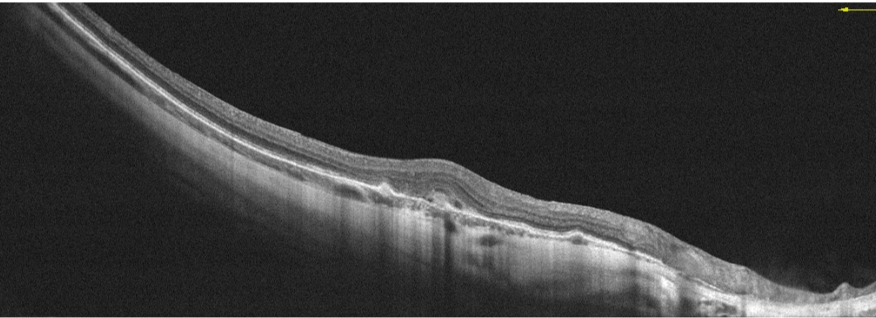
Fovea-centered; Optovue Avanti RTVue XR; optical coherence tomography B-scan — Finding: age-related macular degeneration.